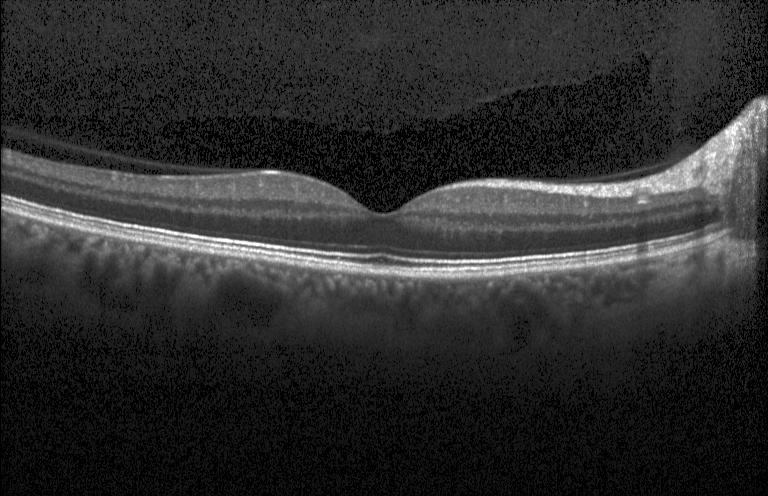

OCT scan showing no choroidal neovascularization, no diabetic macular edema, and no drusen.